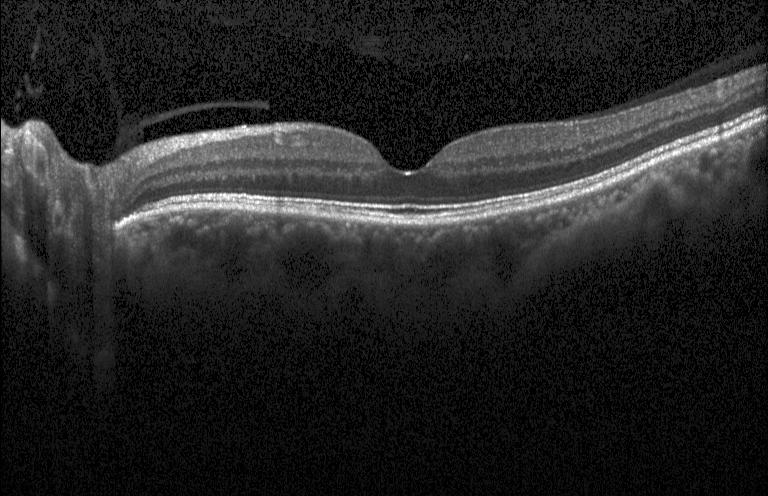 Spectral-domain OCT, Heidelberg Spectralis OCT system, optical coherence tomography scan.
This B-scan demonstrates no CNV, DME, or drusen.